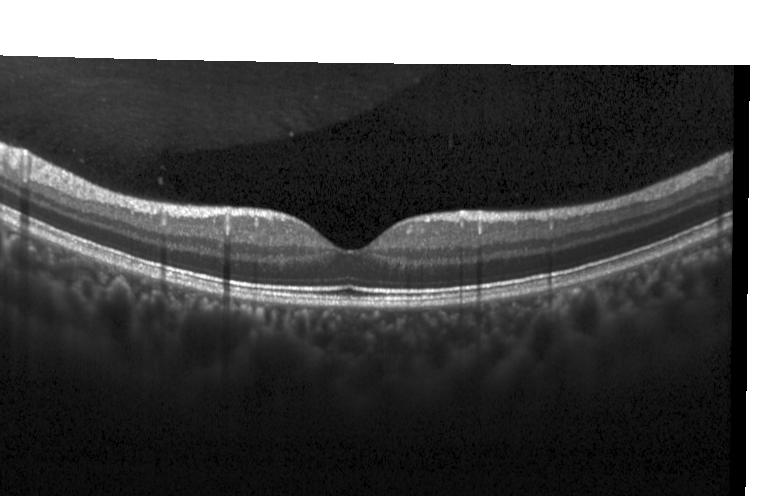
Centered on the fovea · Heidelberg Spectralis OCT system · OCT B-scan. Assessment: no CNV, DME, or drusen.